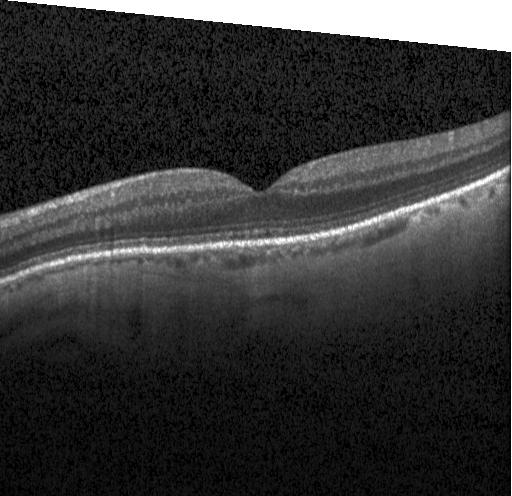
Retinal OCT cross-section showing neither choroidal neovascularization, diabetic macular edema, nor drusen.